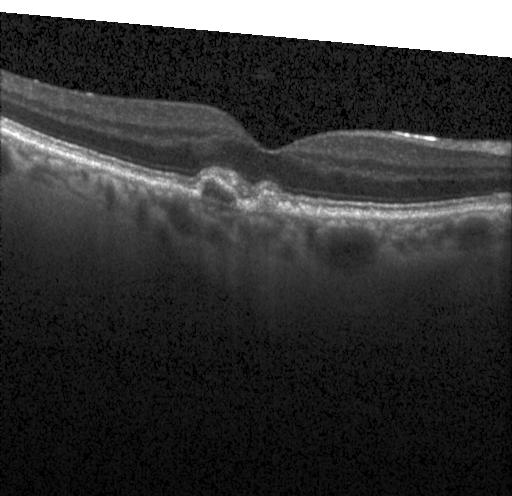

OCT finding: a choroidal neovascular membrane.